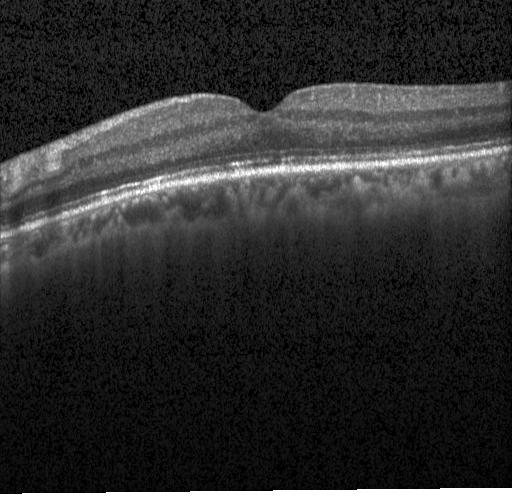
Retinal OCT cross-section showing neither choroidal neovascularization, diabetic macular edema, nor drusen.